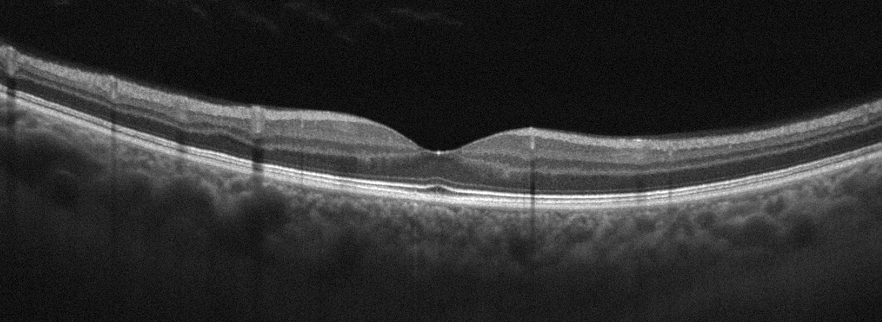

Impression: absence of AMD, DME, ERM, RAO, RVO, and vitreomacular interface disease.